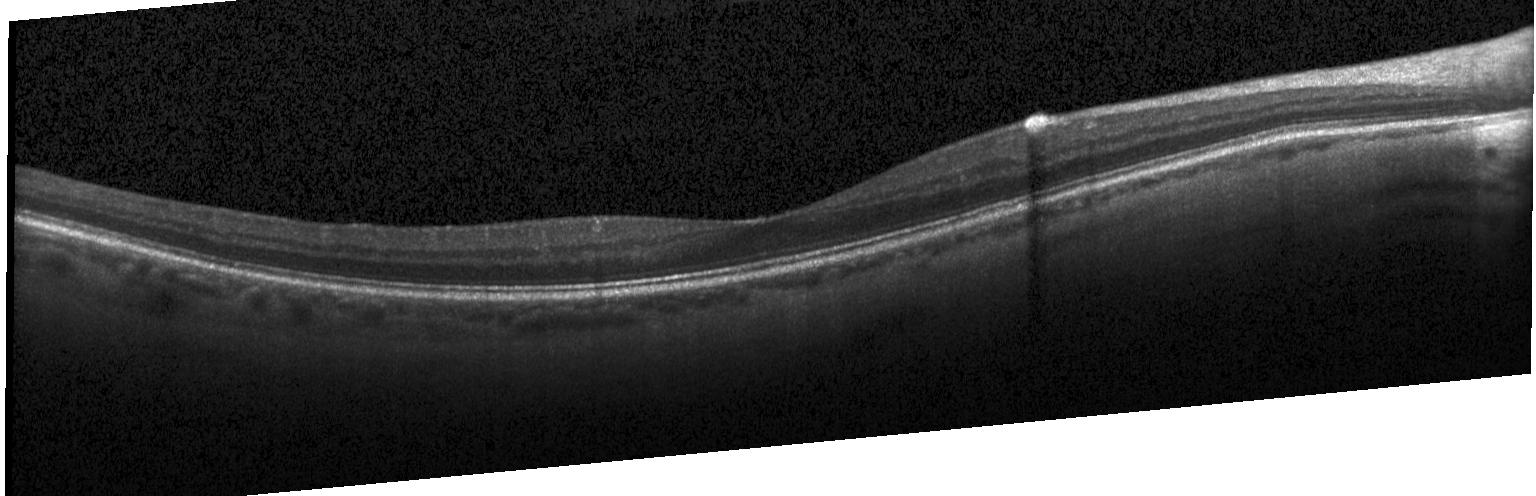 Dx: neither CNV, DME, nor drusen.